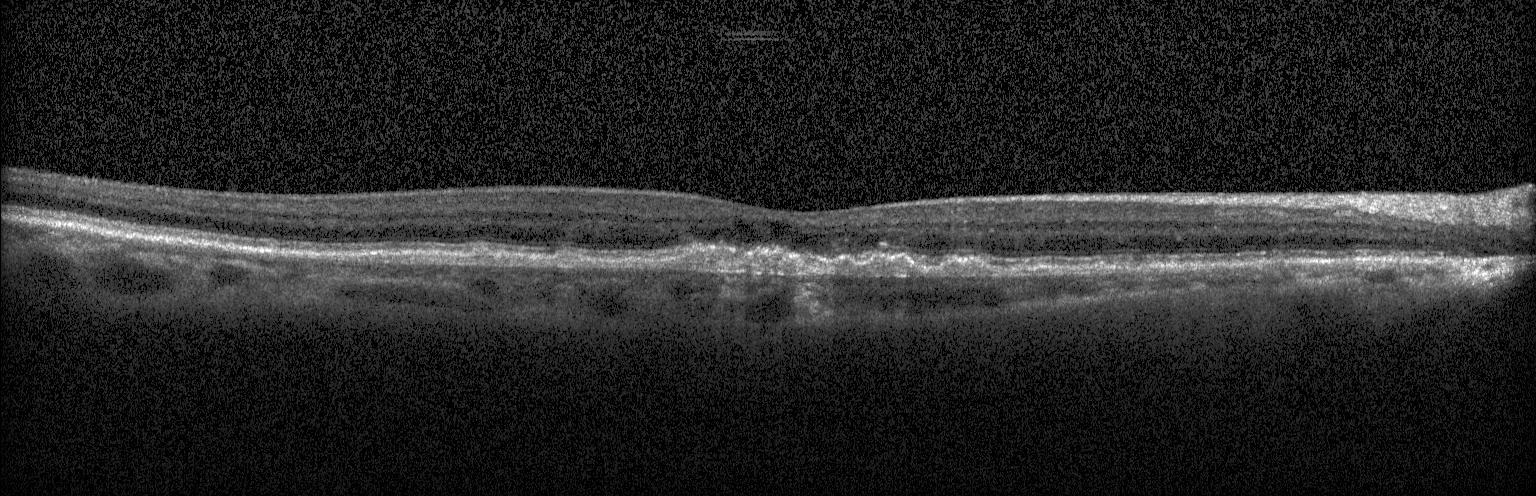
Macular scan · OCT line scan · spectral-domain optical coherence tomography · Heidelberg Spectralis OCT system.
Macular OCT: a choroidal neovascular membrane.